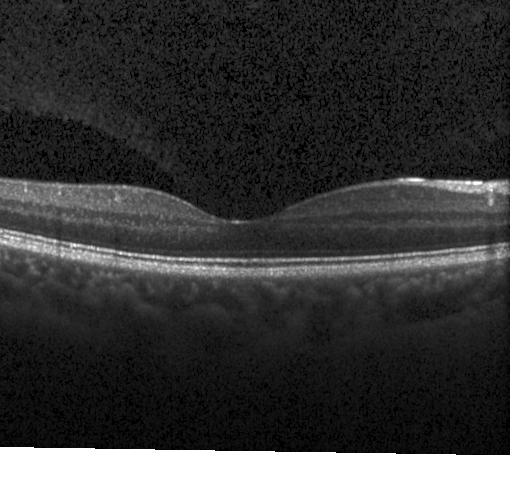

Heidelberg Spectralis OCT system; through the macula; retinal OCT B-scan
Assessment: no evidence of choroidal neovascularization, diabetic macular edema, or drusen.